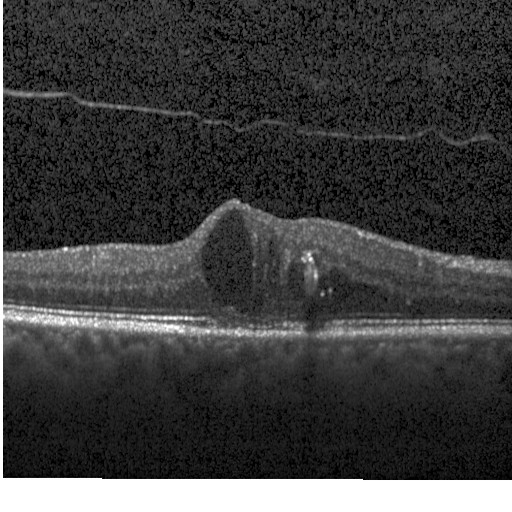 Spectral-domain optical coherence tomography, instrument: Heidelberg Spectralis, OCT line scan, through the macula
Diabetic macular edema.